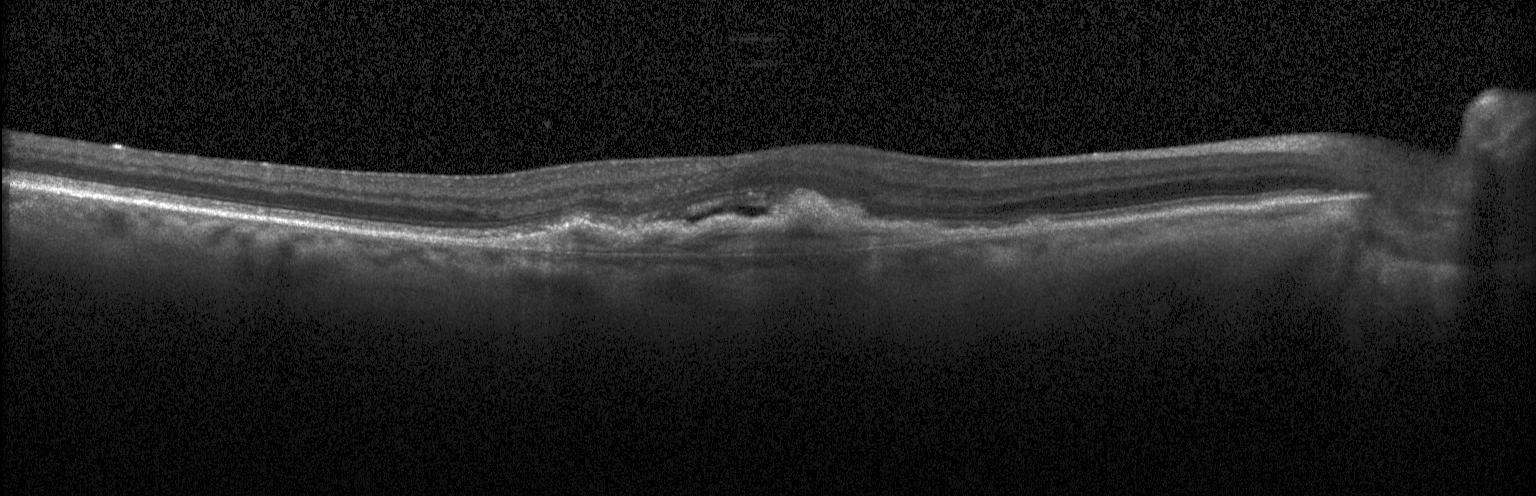

Fovea-centered. OCT B-scan. SD-OCT. Instrument: Heidelberg Spectralis.
This B-scan demonstrates a choroidal neovascular membrane.